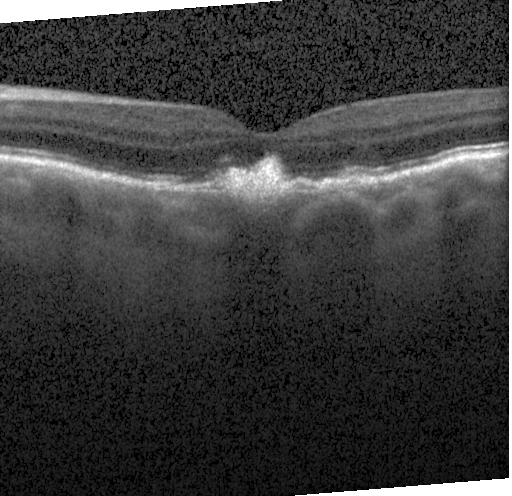

Horizontal scan through the fovea, optical coherence tomography B-scan, SD-OCT — OCT finding: CNV.